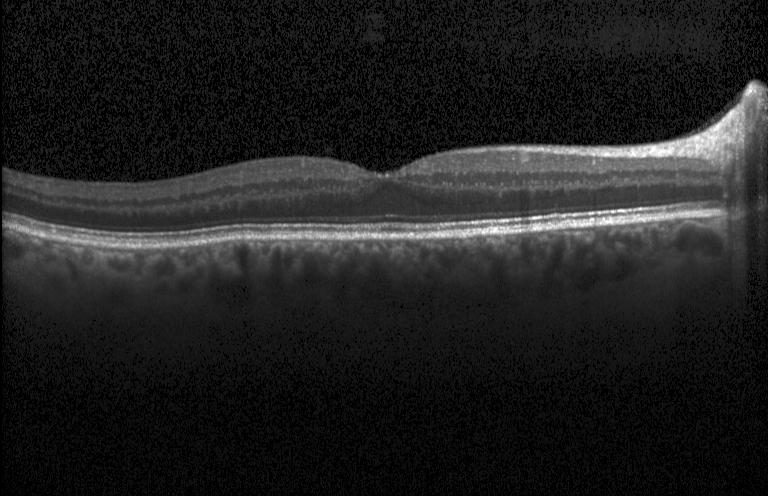 Spectral-domain OCT; optical coherence tomography B-scan. OCT finding: no choroidal neovascularization, no diabetic macular edema, and no drusen.